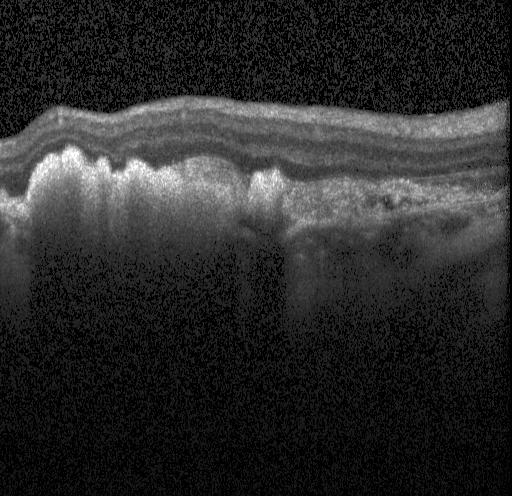

This B-scan demonstrates a choroidal neovascular membrane.